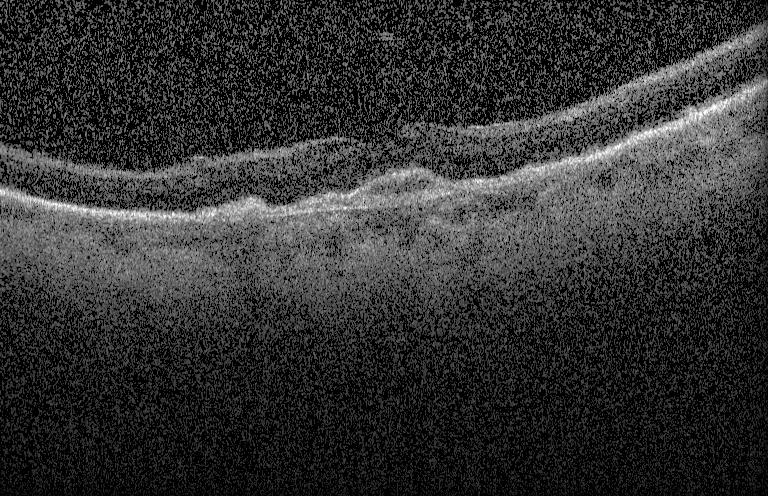

Diagnosis: a choroidal neovascular membrane.